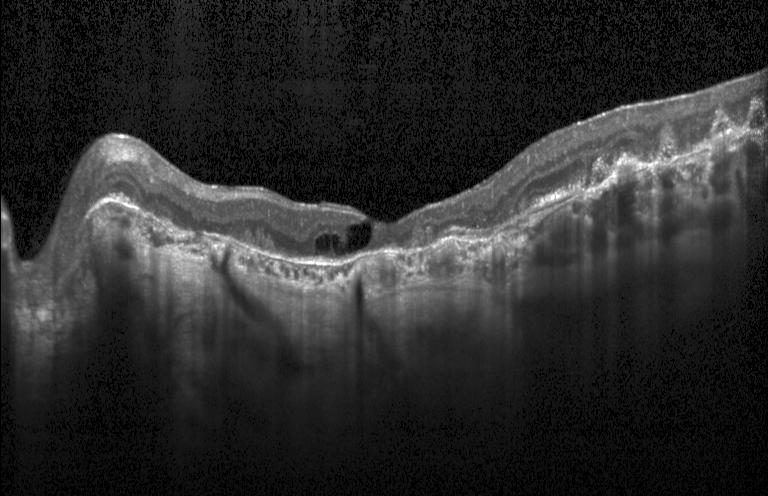
Instrument: Heidelberg Spectralis · spectral-domain optical coherence tomography · horizontal scan through the fovea · optical coherence tomography scan
Dx: choroidal neovascularization.